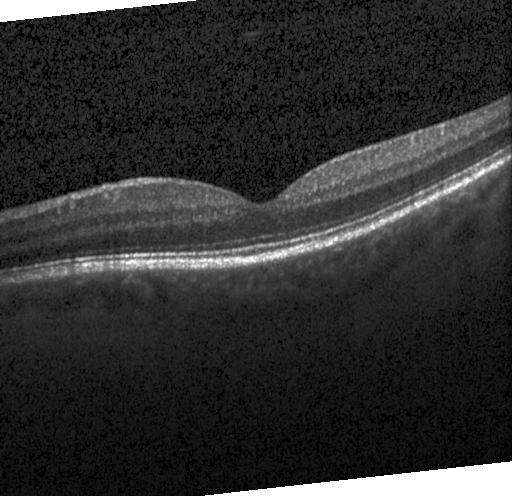

OCT line scan. Impression: no choroidal neovascularization, no diabetic macular edema, and no drusen.